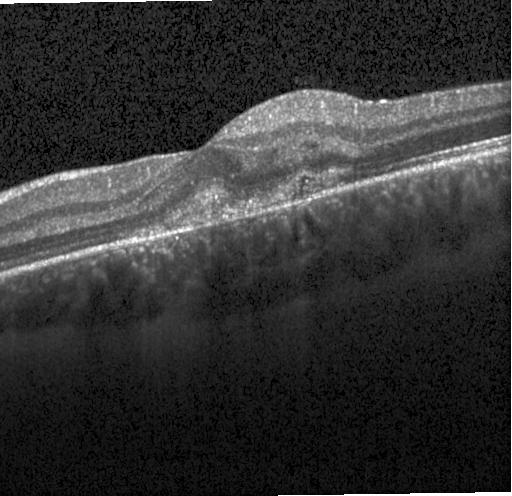 Retinal OCT cross-section showing a choroidal neovascular membrane.